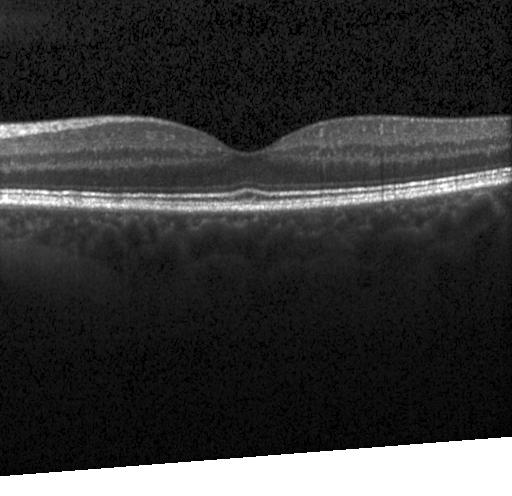

Retinal OCT cross-section — Assessment: no CNV, DME, or drusen.